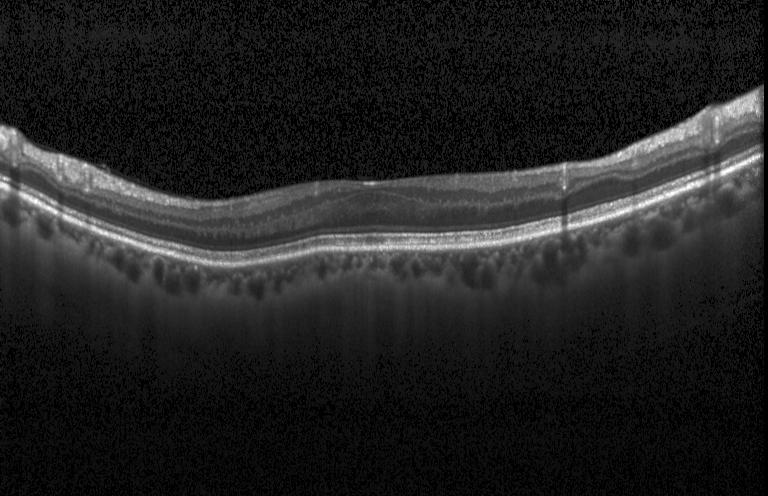
Impression: neither choroidal neovascularization, diabetic macular edema, nor drusen.